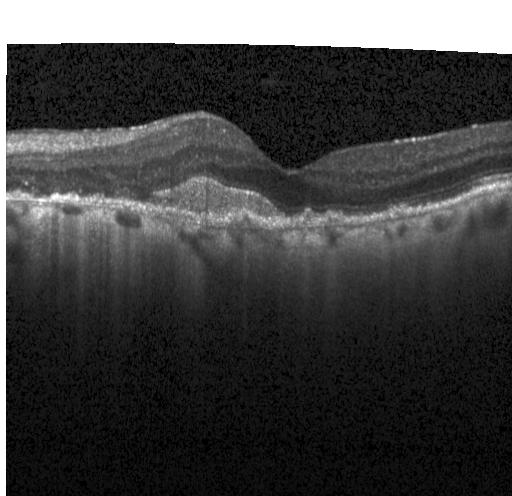
Instrument: Heidelberg Spectralis; retinal OCT B-scan. Impression: a choroidal neovascular membrane.